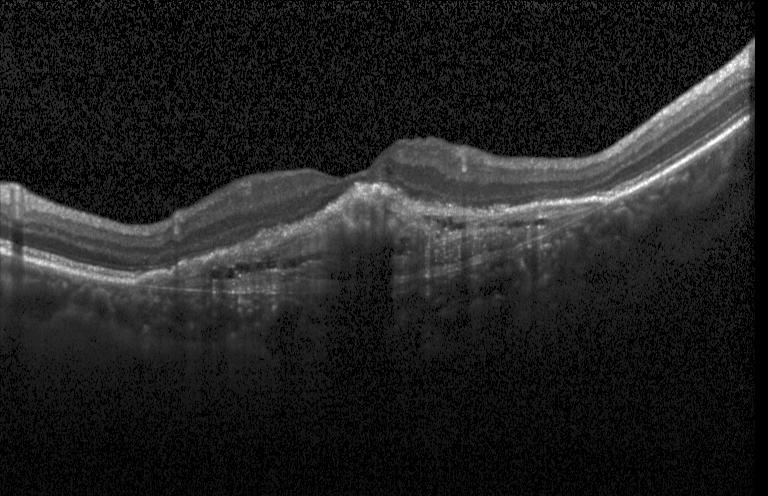

Diagnosis: choroidal neovascularization (CNV).